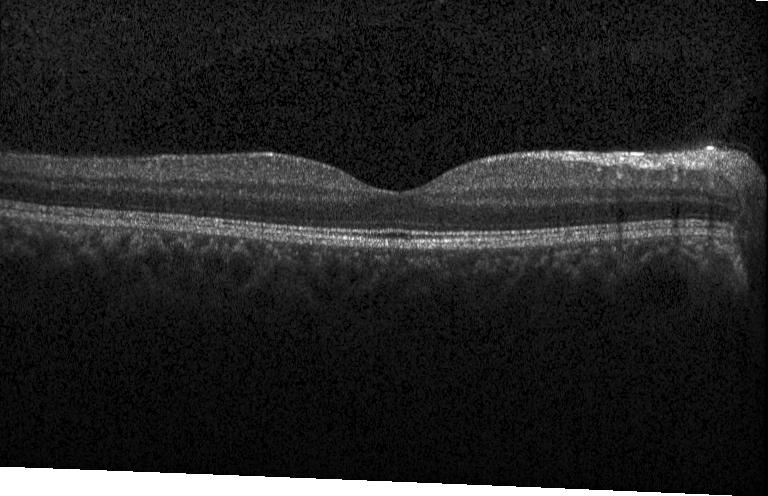 Spectral-domain optical coherence tomography · optical coherence tomography scan. Dx: no CNV, no DME, and no drusen.